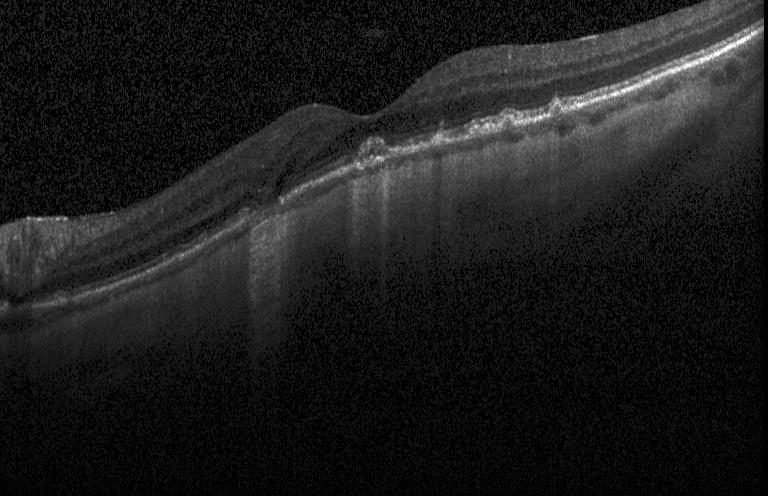
Fovea-centered; spectral-domain OCT; OCT line scan; acquired on a Heidelberg Spectralis.
OCT finding: choroidal neovascularization.